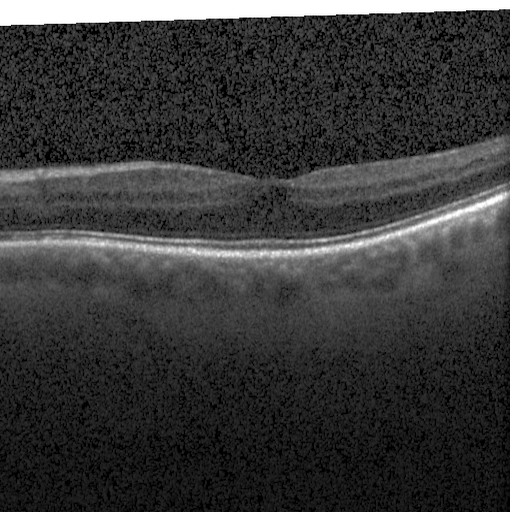

Retinal OCT B-scan, Heidelberg Spectralis OCT system, spectral-domain optical coherence tomography, horizontal scan through the fovea
Diagnosis: DME.